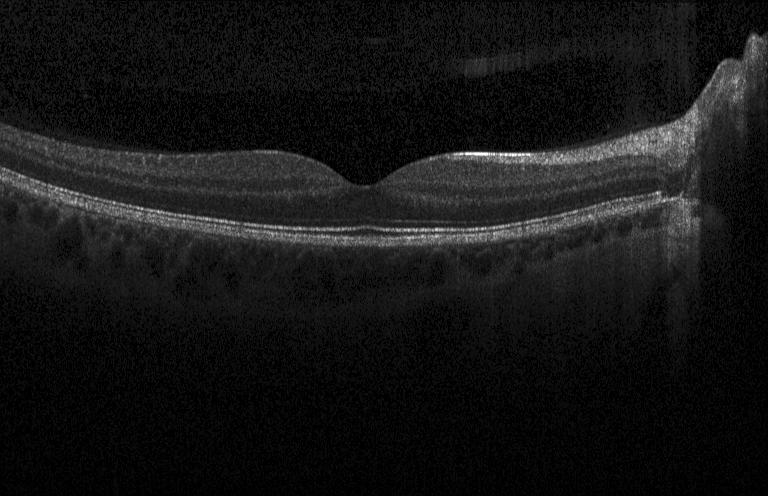

Macular OCT: no choroidal neovascularization, no diabetic macular edema, and no drusen.